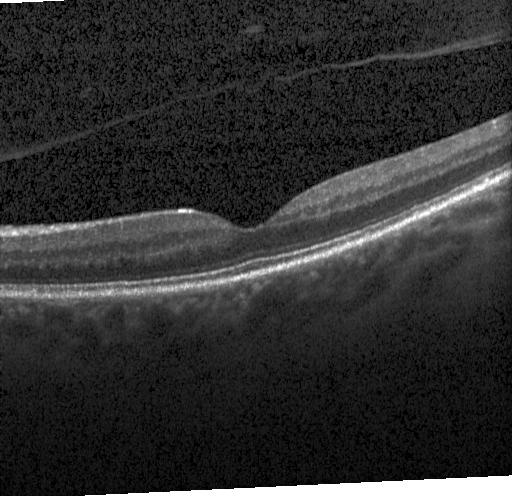

Heidelberg Spectralis OCT system. Retinal OCT B-scan.
Impression: neither choroidal neovascularization, diabetic macular edema, nor drusen.